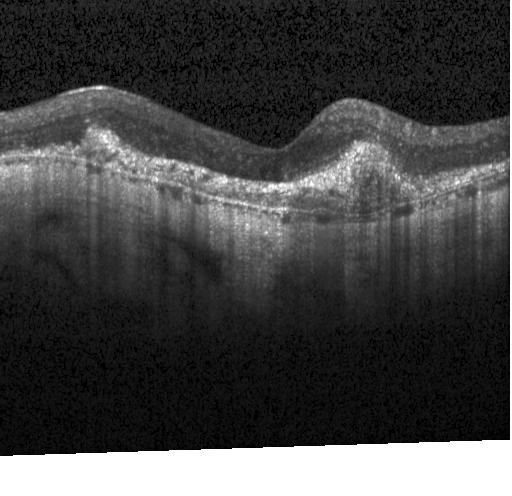

Macular OCT: a choroidal neovascular membrane.